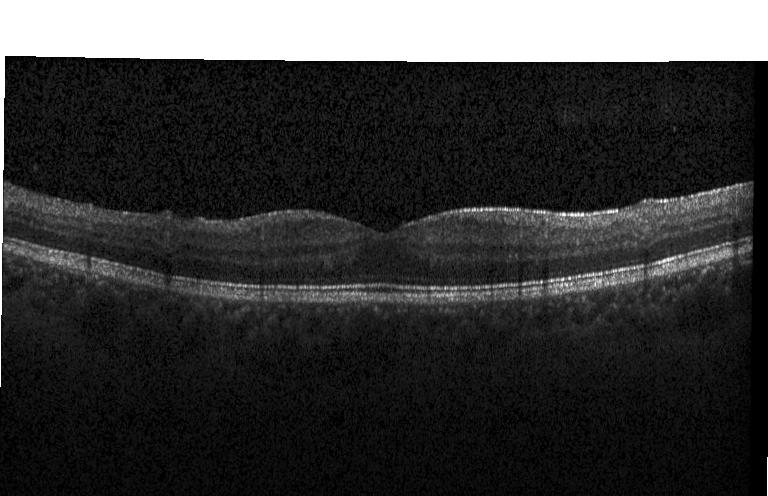
Optical coherence tomography scan. Assessment: no choroidal neovascularization, diabetic macular edema, or drusen.